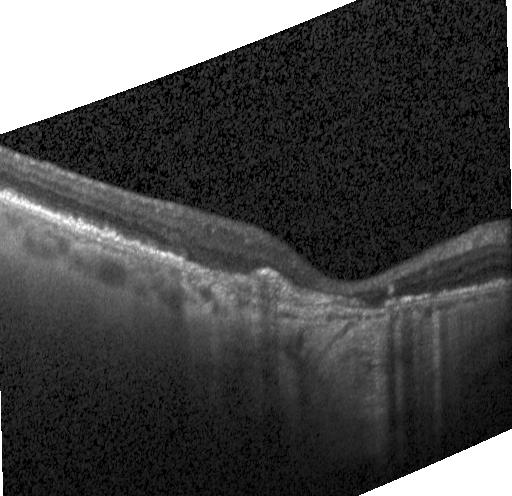
Macular OCT: a choroidal neovascular membrane.